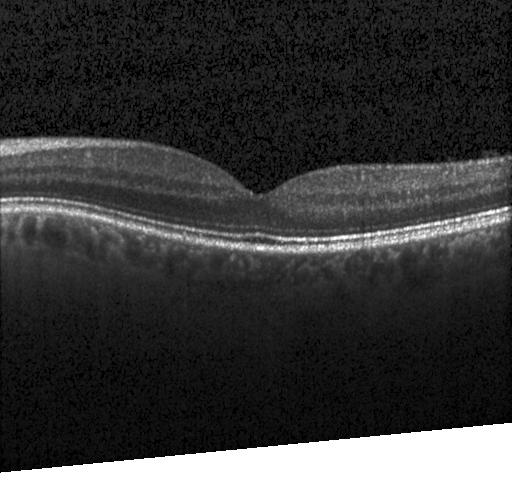 Acquired on a Heidelberg Spectralis · OCT line scan · spectral-domain OCT · horizontal scan through the fovea — The scan shows no CNV, no DME, and no drusen.